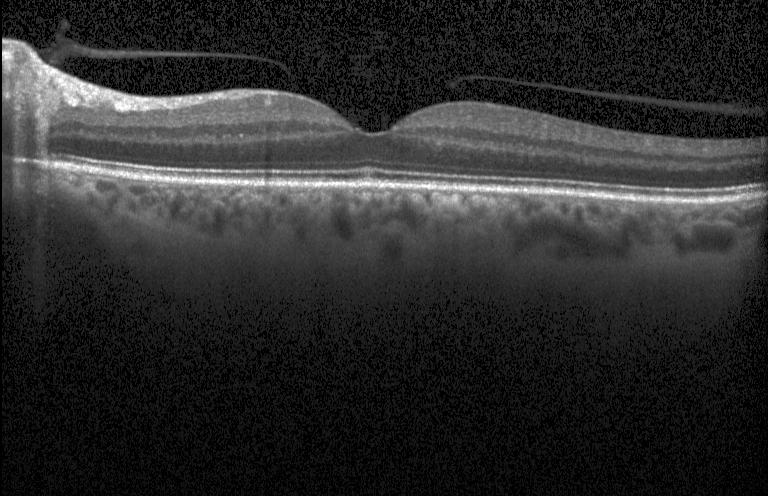 Heidelberg Spectralis. Spectral-domain OCT. OCT B-scan
Macular OCT: no evidence of choroidal neovascularization, diabetic macular edema, or drusen.